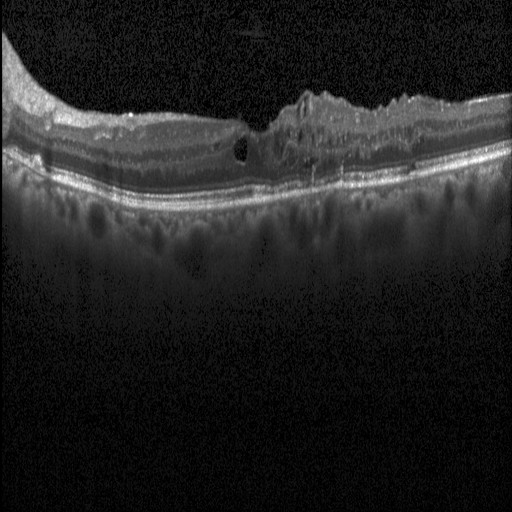
Macular OCT: DME.